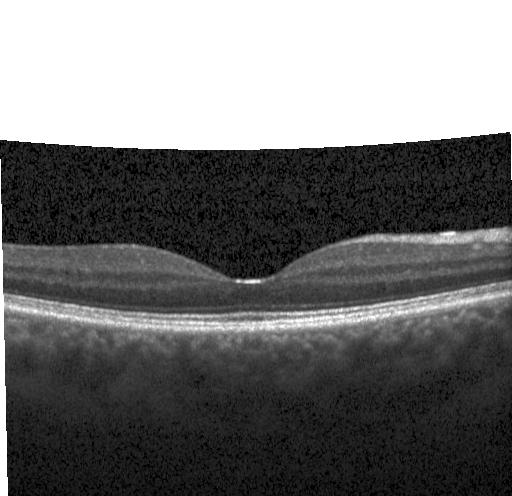 No evidence of CNV, DME, or drusen.